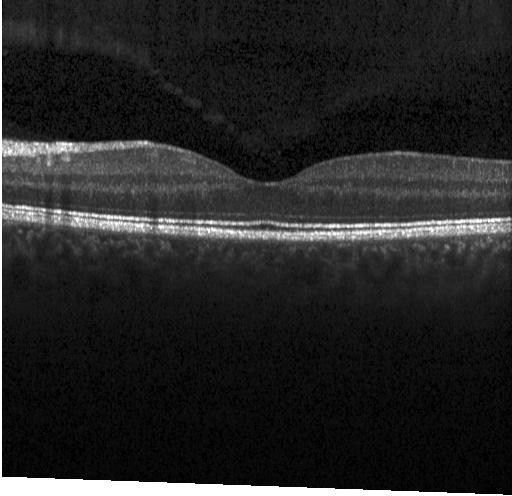

Optical coherence tomography B-scan, spectral-domain optical coherence tomography, horizontal scan through the fovea, Heidelberg Spectralis — Finding: no CNV, no DME, and no drusen.